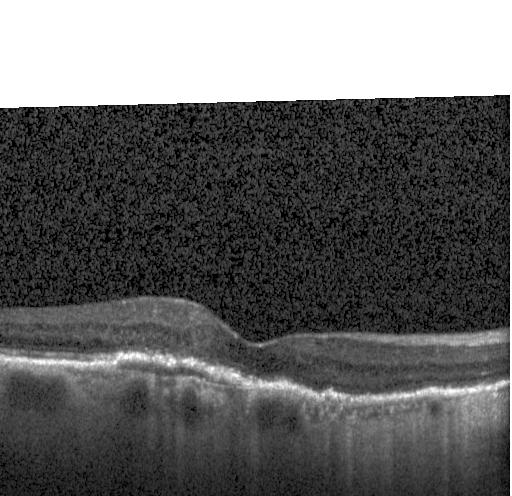

Impression: choroidal neovascularization.